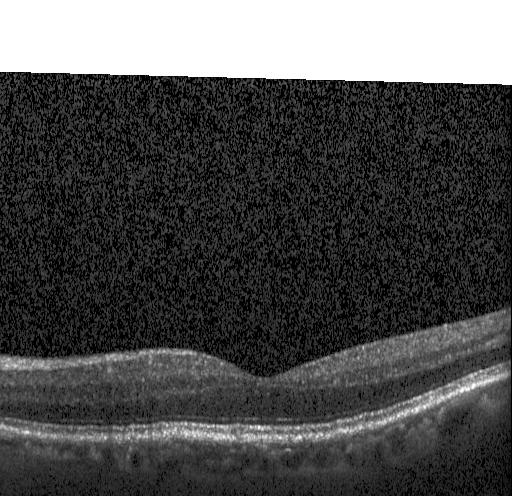

Impression: no choroidal neovascularization, no diabetic macular edema, and no drusen.